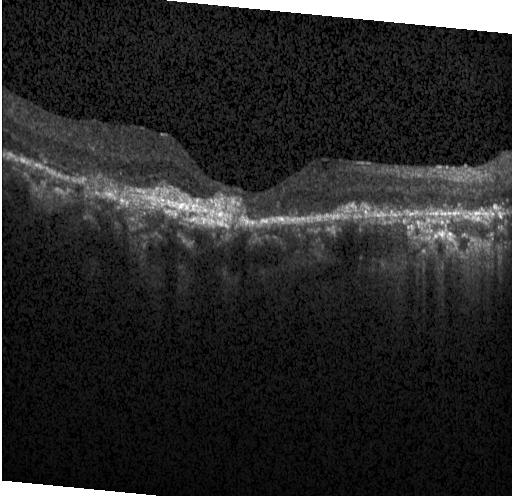 Retinal OCT B-scan, spectral-domain OCT.
Dx: a choroidal neovascular membrane.